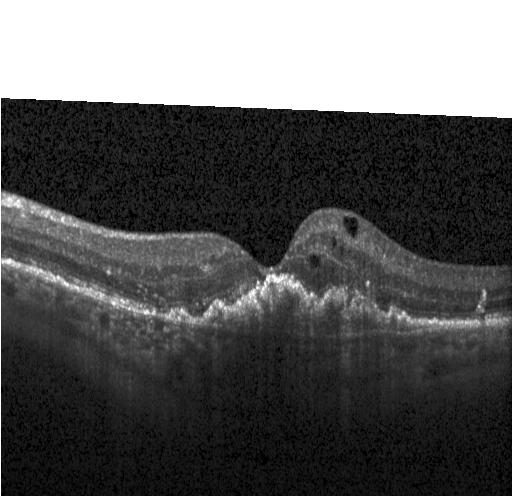 Retinal OCT cross-section showing a choroidal neovascular membrane.